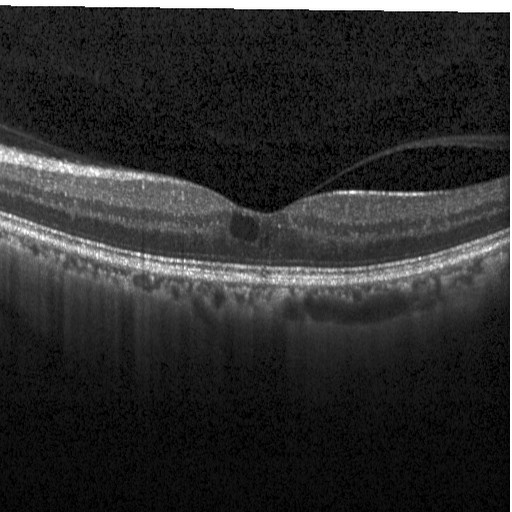

Spectral-domain OCT · through the macula · retinal OCT B-scan. Dx: diabetic macular edema.